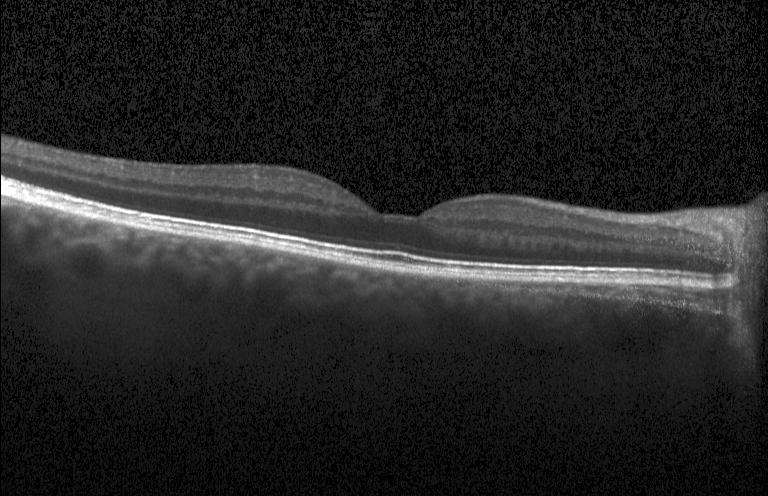 Heidelberg Spectralis OCT system, centered on the fovea, optical coherence tomography scan.
Finding: no CNV, no DME, and no drusen.